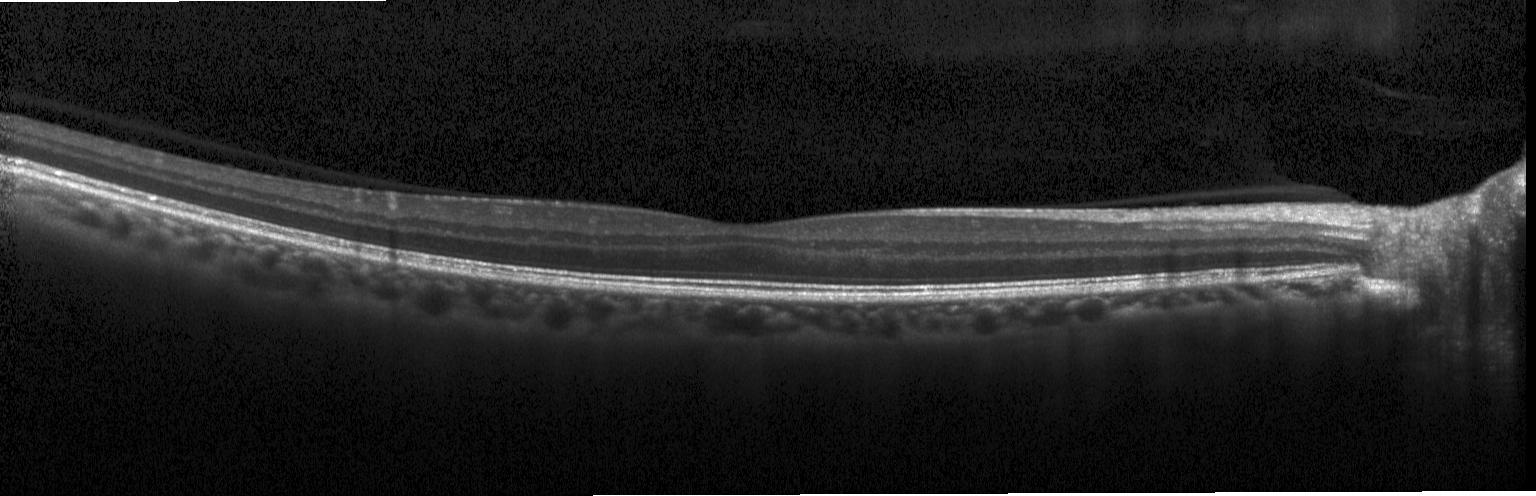
OCT line scan. Assessment: no choroidal neovascularization, diabetic macular edema, or drusen.